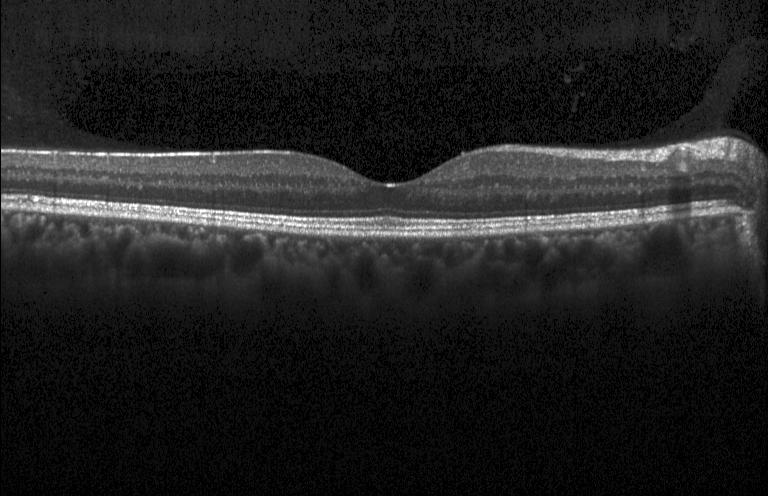

OCT line scan
This B-scan demonstrates neither CNV, DME, nor drusen.